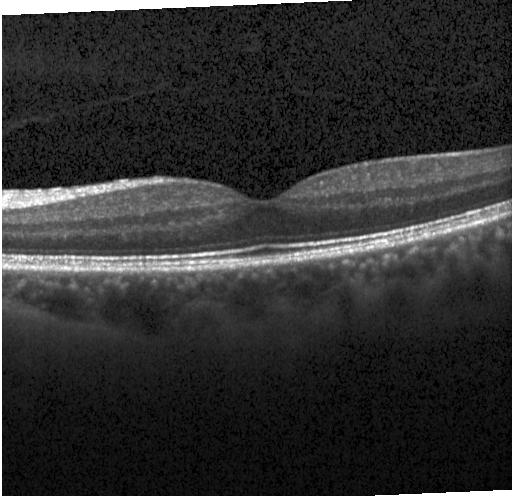
Diagnosis: neither choroidal neovascularization, diabetic macular edema, nor drusen.